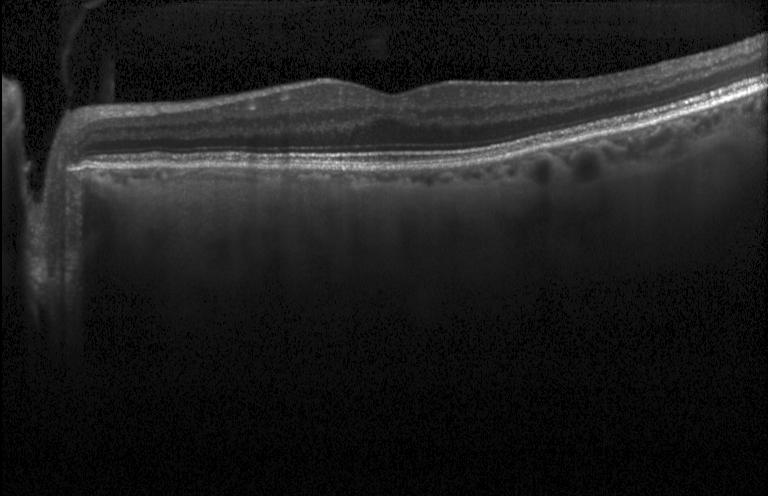
Retinal OCT cross-section.
No CNV, DME, or drusen.